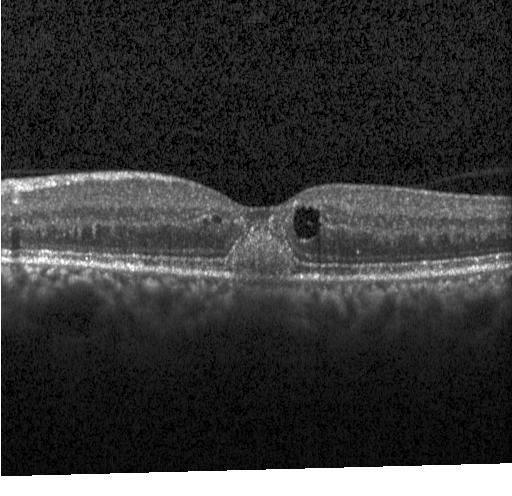
OCT line scan — Assessment: a choroidal neovascular membrane.